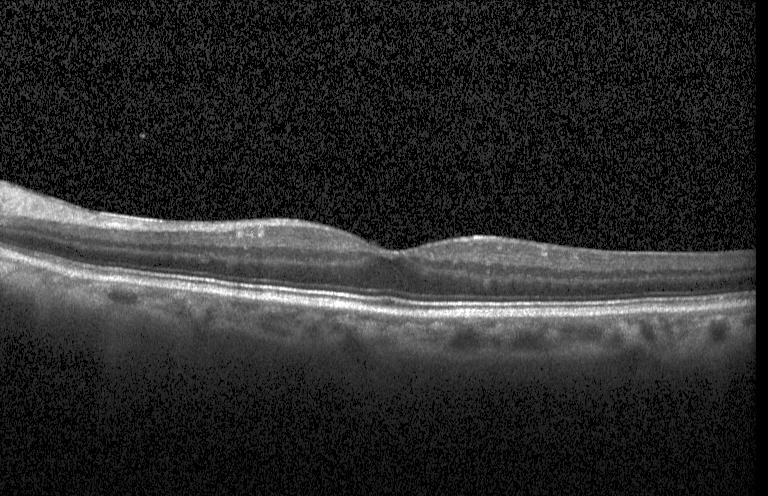 Macular OCT: neither choroidal neovascularization, diabetic macular edema, nor drusen.